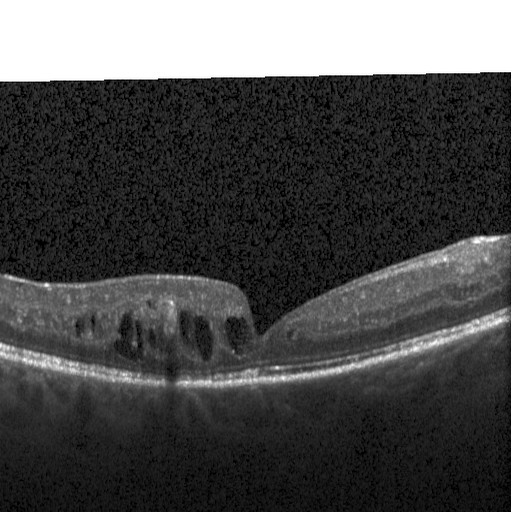 OCT B-scan showing diabetic macular edema.